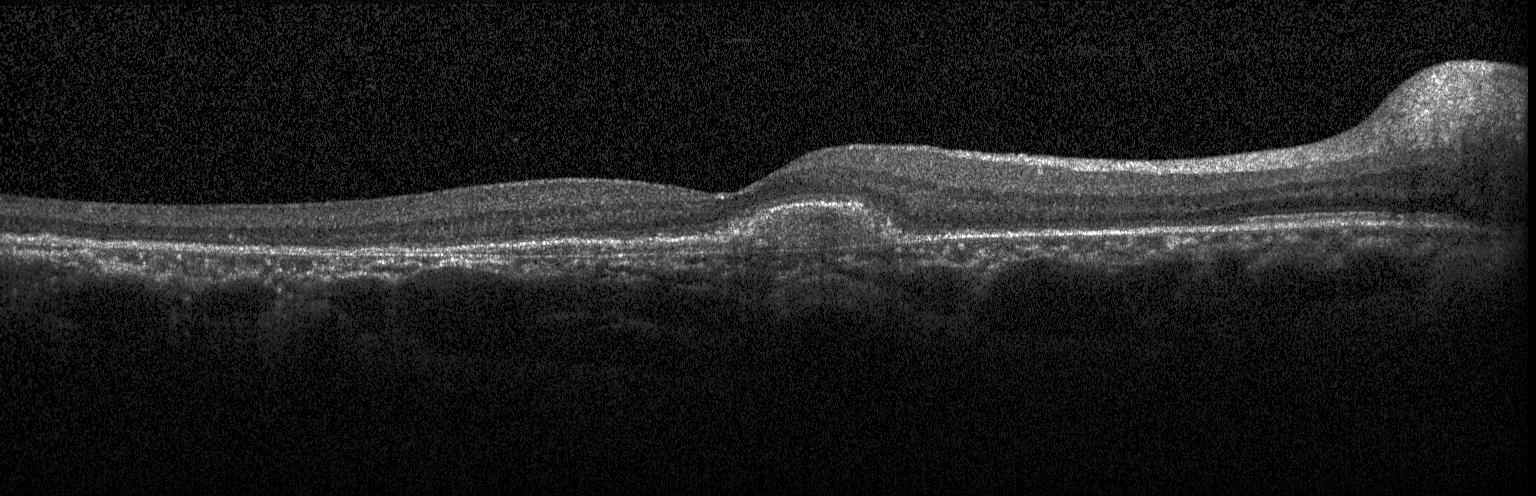 Impression: a choroidal neovascular membrane.